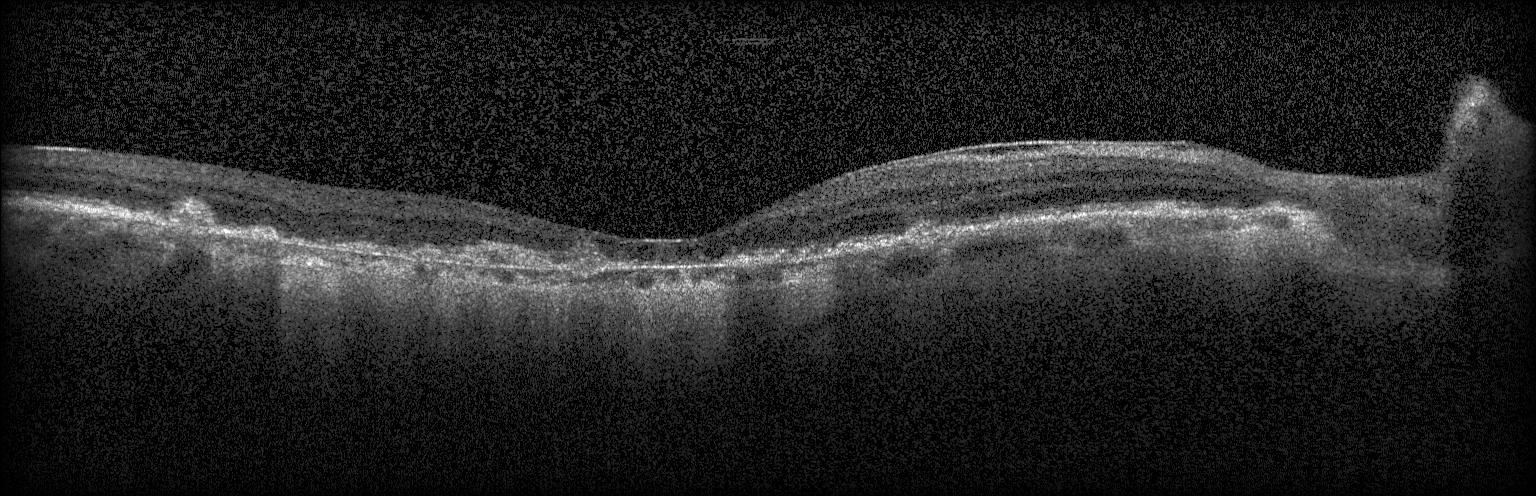 Spectral-domain OCT, OCT B-scan, through the macula, instrument: Heidelberg Spectralis
OCT finding: a choroidal neovascular membrane.